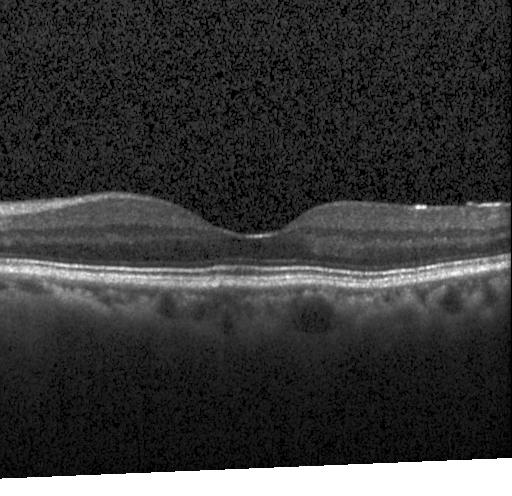
Spectral-domain OCT B-scan: no evidence of choroidal neovascularization, diabetic macular edema, or drusen.